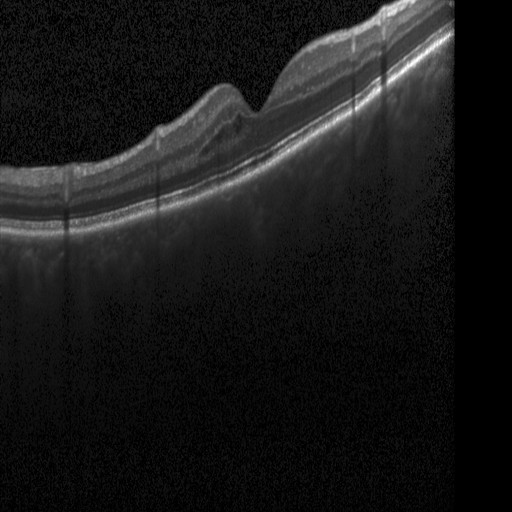 OCT scan showing diabetic macular edema (DME).